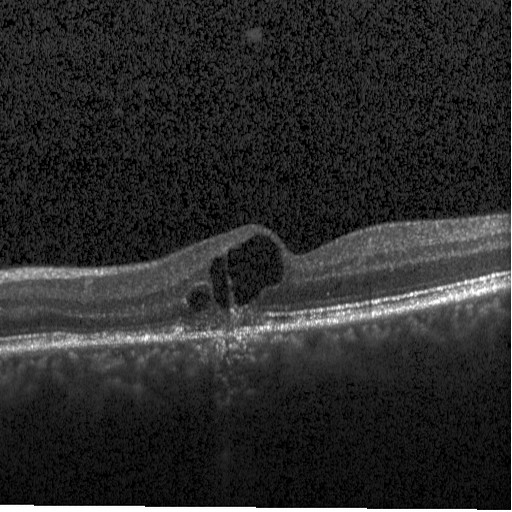
The scan shows diabetic macular edema (DME).